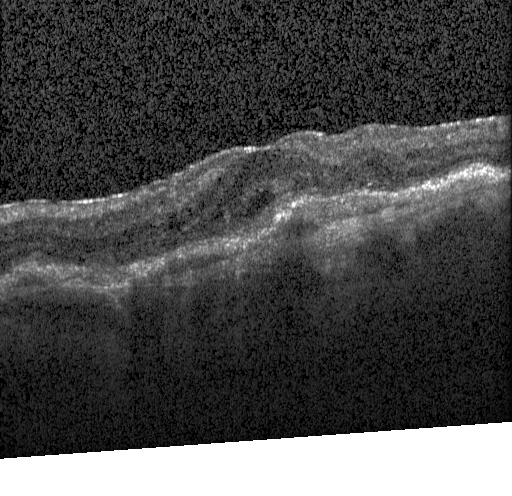 Retinal OCT B-scan. OCT finding: choroidal neovascularization (CNV).